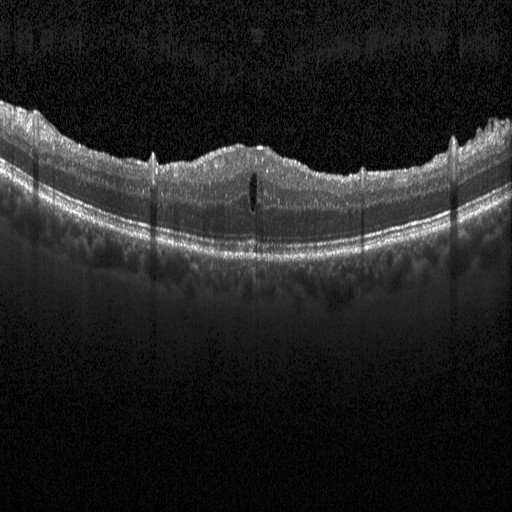
Optical coherence tomography B-scan · horizontal scan through the fovea · spectral-domain OCT · Heidelberg Spectralis.
OCT finding: diabetic macular edema (DME).